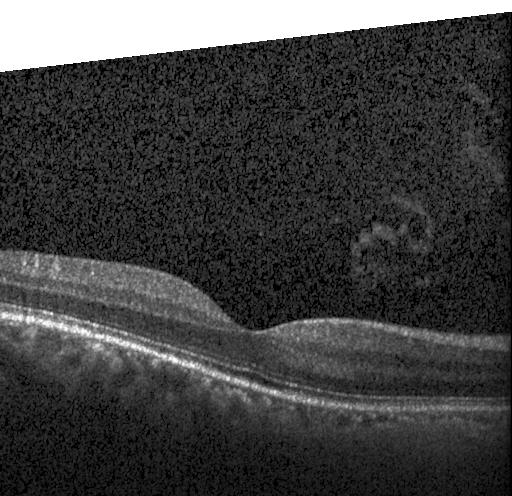
Fovea-centered. Retinal OCT cross-section. Spectral-domain optical coherence tomography. Heidelberg Spectralis OCT system. OCT finding: no CNV, DME, or drusen.